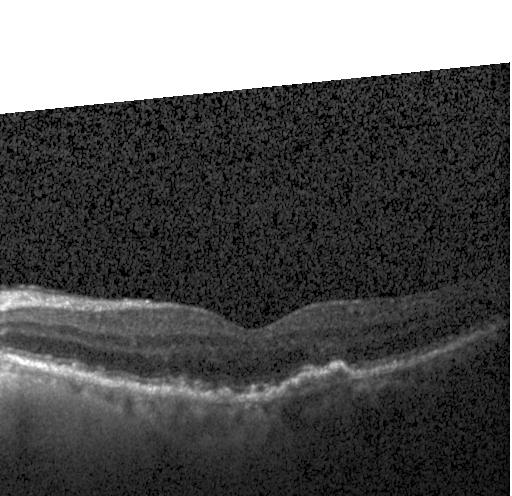 Dx: a choroidal neovascular membrane.